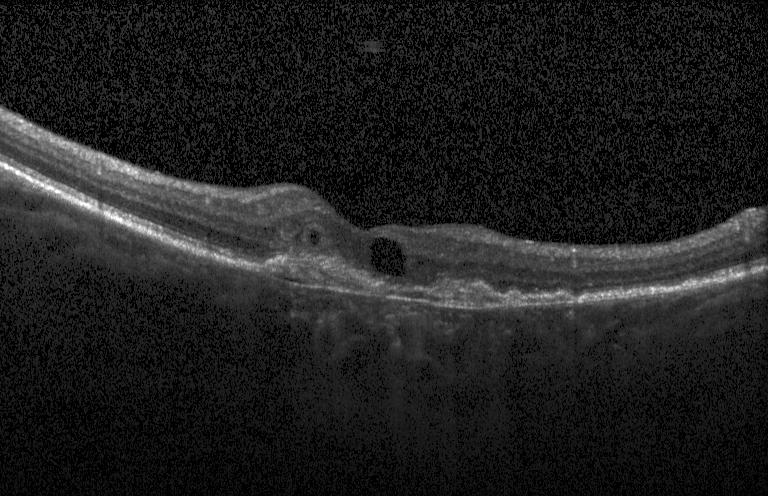

Retinal OCT B-scan — Impression: choroidal neovascularization.